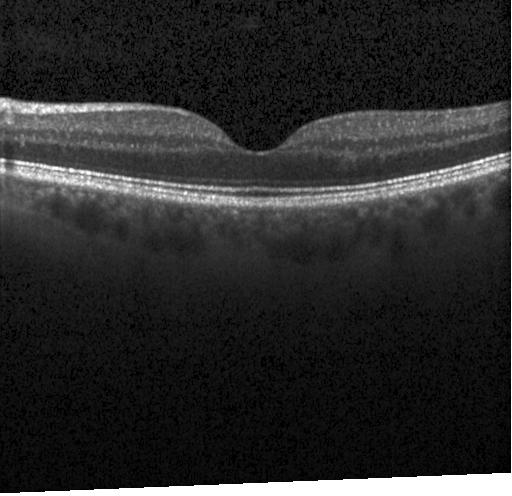
OCT B-scan; centered on the fovea.
Finding: no choroidal neovascularization, no diabetic macular edema, and no drusen.